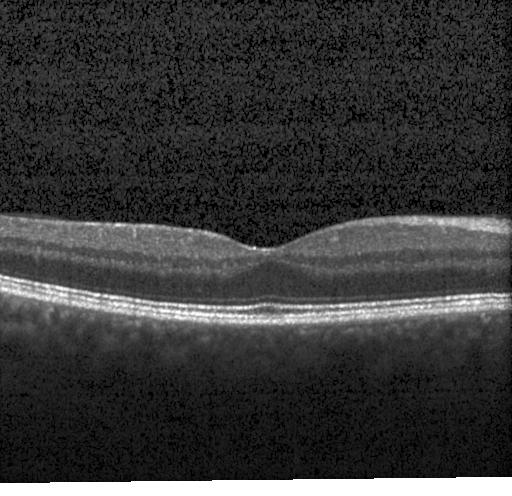

Through the macula; OCT line scan.
Diagnosis: no evidence of choroidal neovascularization, diabetic macular edema, or drusen.